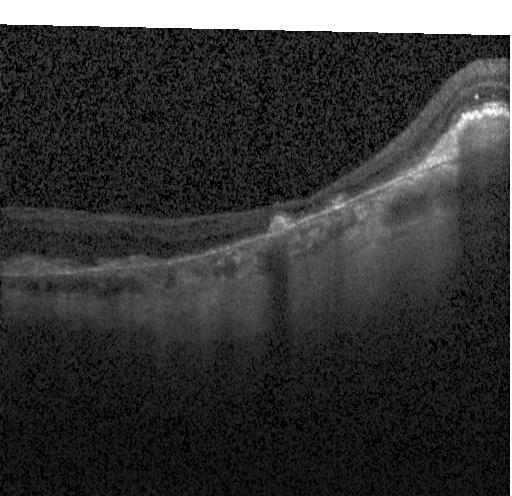
Retinal OCT cross-section.
Diagnosis: choroidal neovascularization.